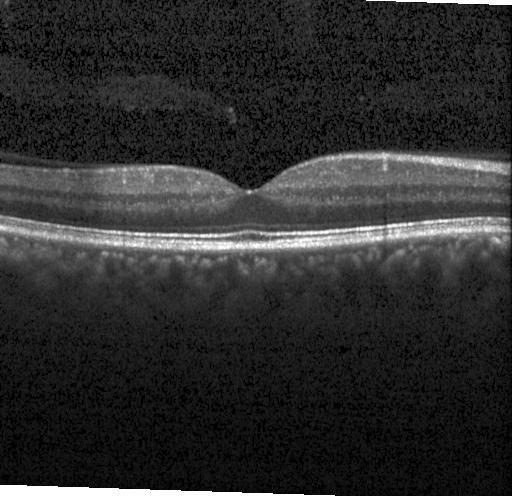

Fovea-centered; spectral-domain OCT; retinal OCT B-scan; instrument: Heidelberg Spectralis. No CNV, no DME, and no drusen.